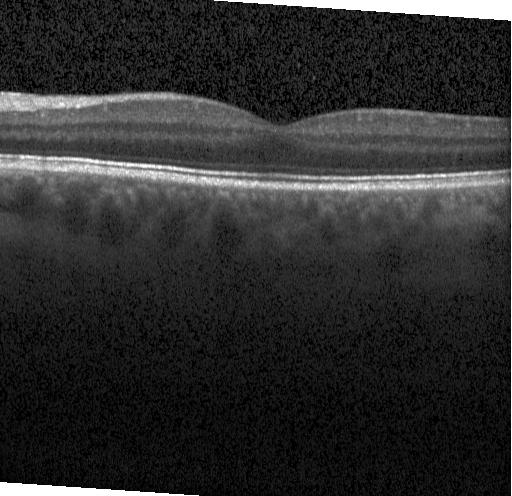 OCT B-scan.
Diagnosis: no evidence of CNV, DME, or drusen.